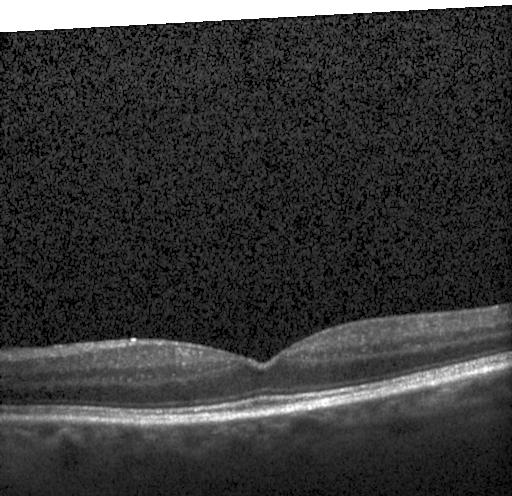

SD-OCT; optical coherence tomography scan; horizontal scan through the fovea
Macular OCT: no choroidal neovascularization, diabetic macular edema, or drusen.